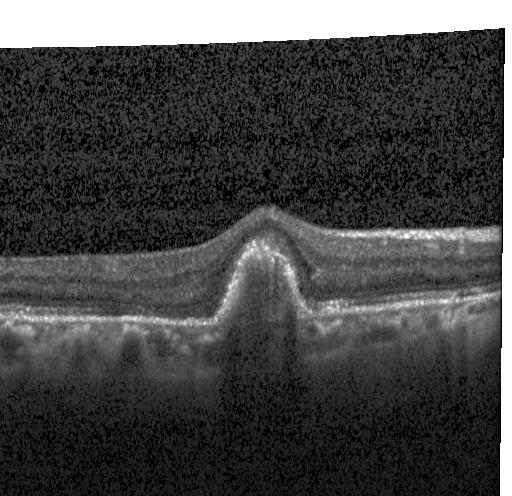 Fovea-centered · instrument: Heidelberg Spectralis · retinal OCT cross-section.
The scan shows a choroidal neovascular membrane.